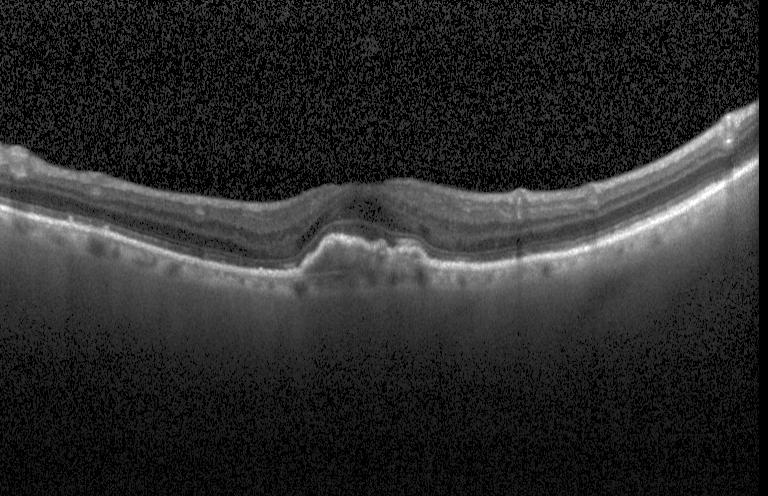

Assessment: a choroidal neovascular membrane.